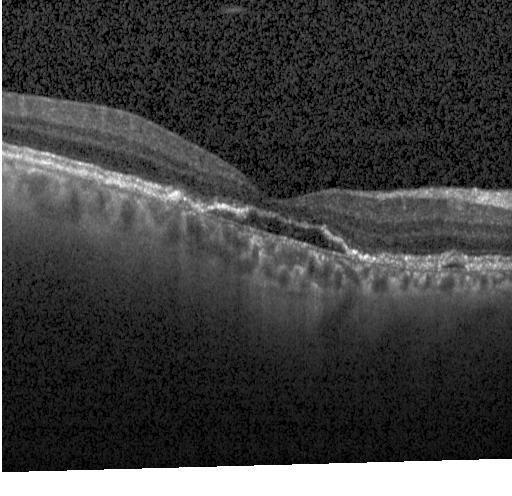 Optical coherence tomography scan.
Finding: choroidal neovascularization (CNV).